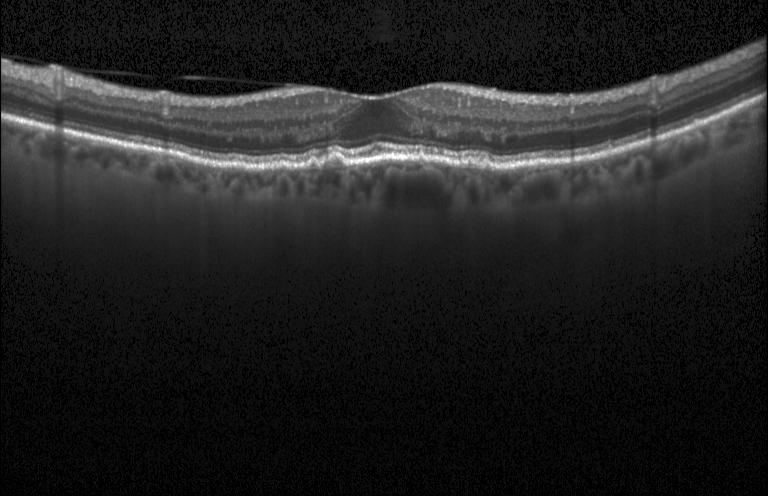
Macular OCT: drusen.